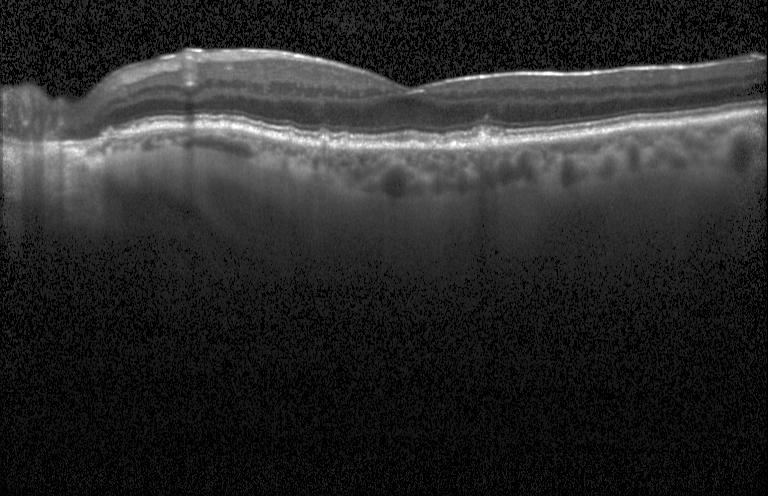 SD-OCT; optical coherence tomography scan; fovea-centered
Impression: multiple drusen.